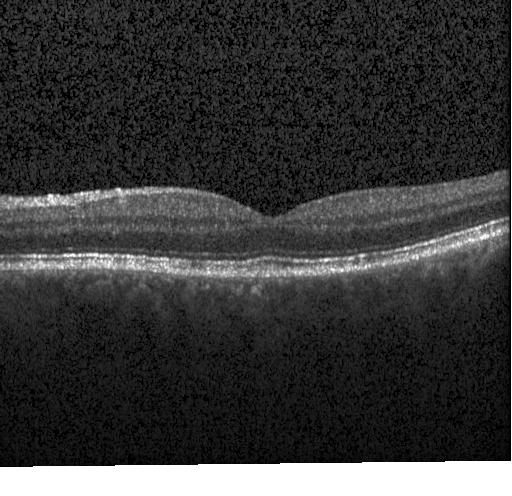
Spectral-domain OCT B-scan: no evidence of choroidal neovascularization, diabetic macular edema, or drusen.